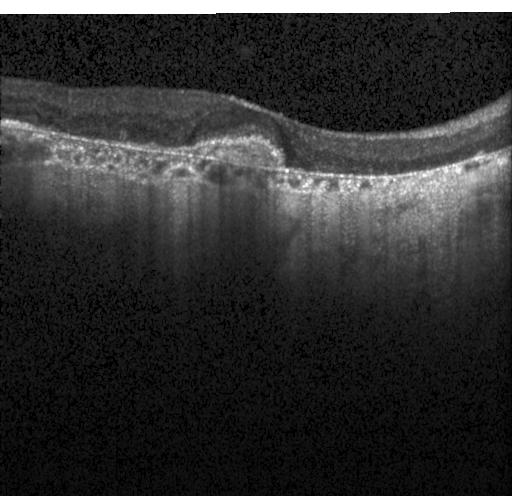
OCT line scan · spectral-domain optical coherence tomography. Impression: a choroidal neovascular membrane.